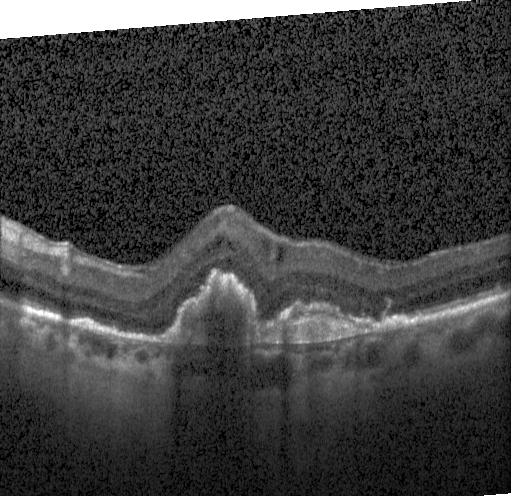
Optical coherence tomography scan; spectral-domain OCT; macular scan; instrument: Heidelberg Spectralis. Macular OCT: a choroidal neovascular membrane.